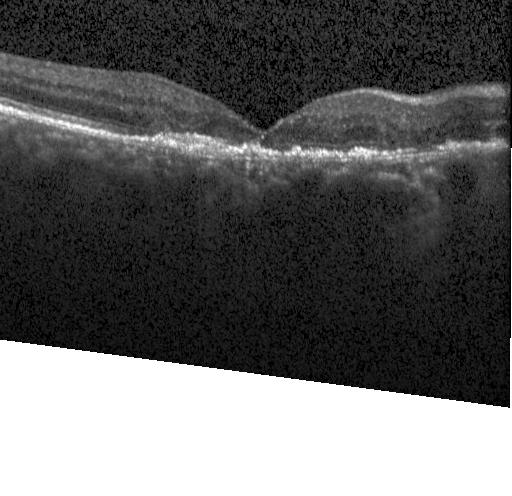
Heidelberg Spectralis. Retinal OCT B-scan — Finding: choroidal neovascularization (CNV).